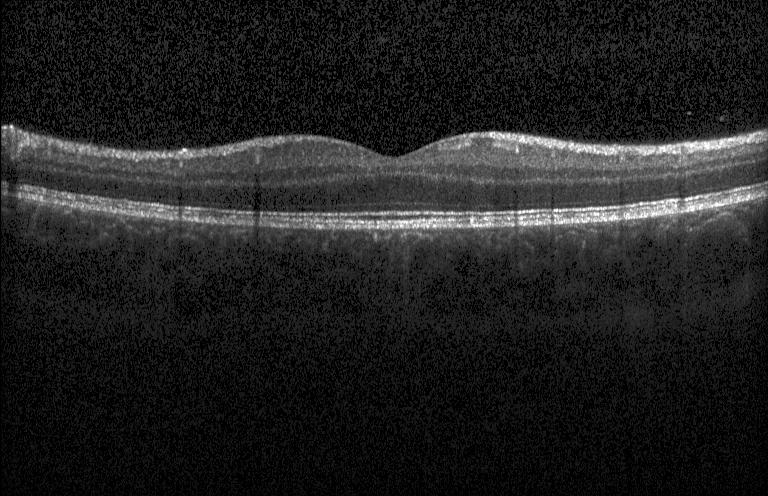 Optical coherence tomography B-scan. This B-scan demonstrates no evidence of choroidal neovascularization, diabetic macular edema, or drusen.